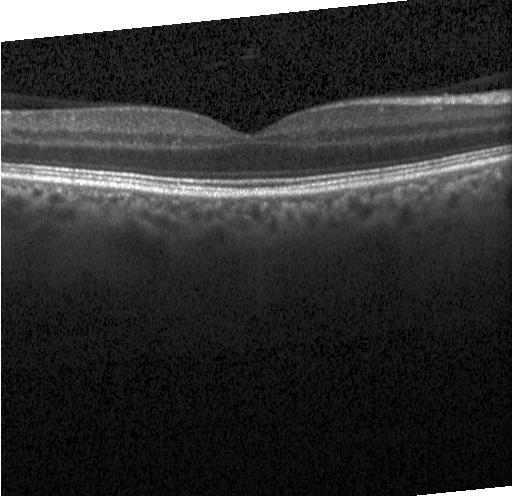

Spectral-domain OCT; optical coherence tomography scan.
OCT finding: no choroidal neovascularization, no diabetic macular edema, and no drusen.